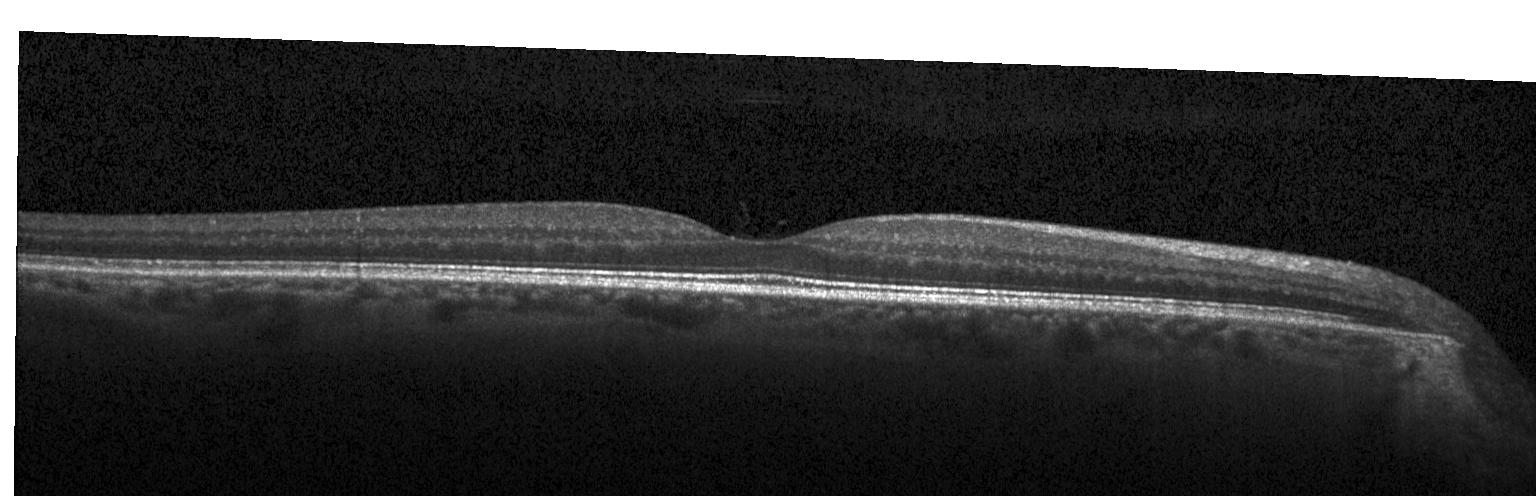

Impression: neither choroidal neovascularization, diabetic macular edema, nor drusen.